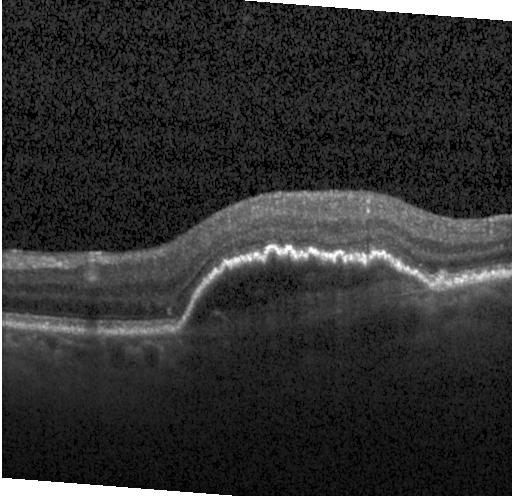
Acquired on a Heidelberg Spectralis, OCT line scan — Diagnosis: a choroidal neovascular membrane.